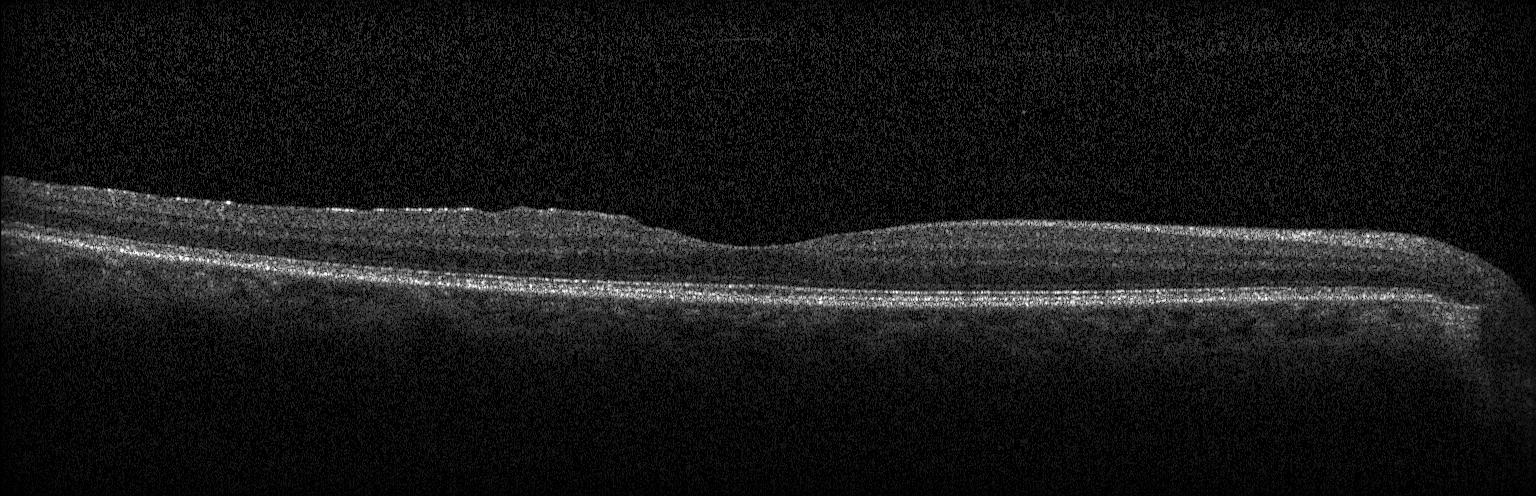

Optical coherence tomography B-scan.
This B-scan demonstrates no CNV, DME, or drusen.